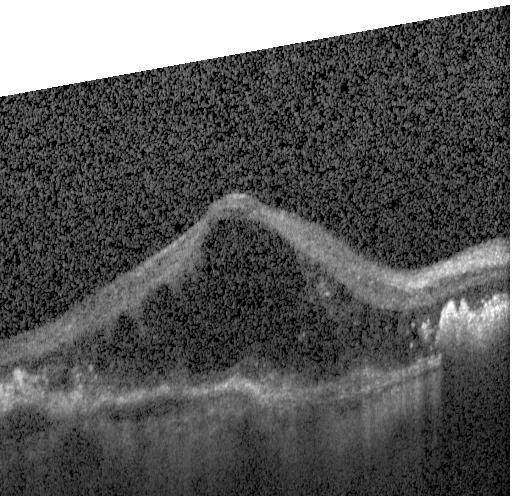
Fovea-centered; Heidelberg Spectralis; optical coherence tomography scan. CNV.